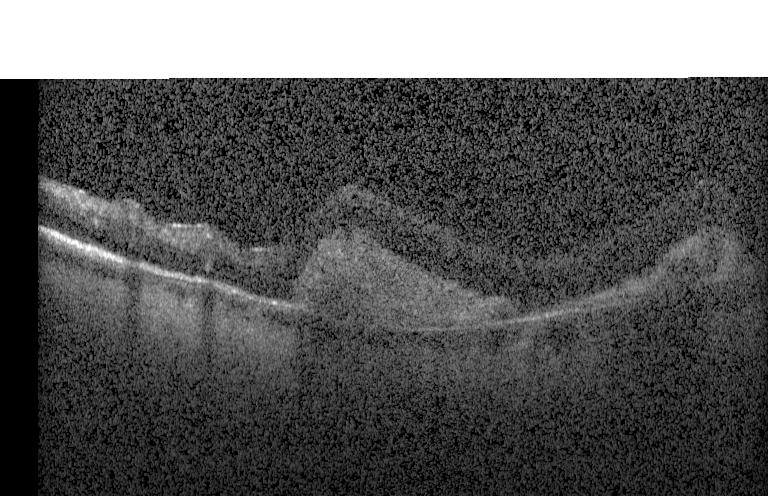 Retinal OCT B-scan. Acquired on a Heidelberg Spectralis.
Macular OCT: a choroidal neovascular membrane.